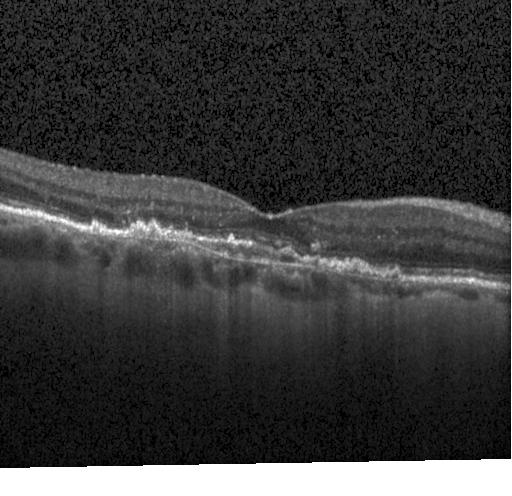

Impression: a choroidal neovascular membrane.